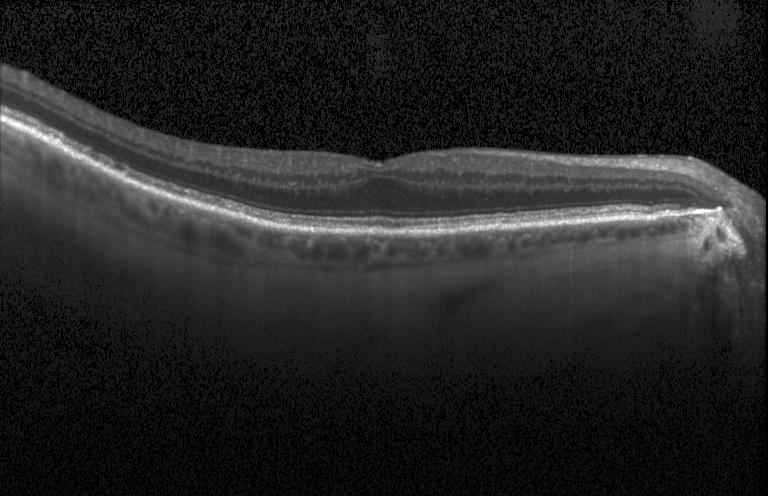

The scan shows neither choroidal neovascularization, diabetic macular edema, nor drusen.